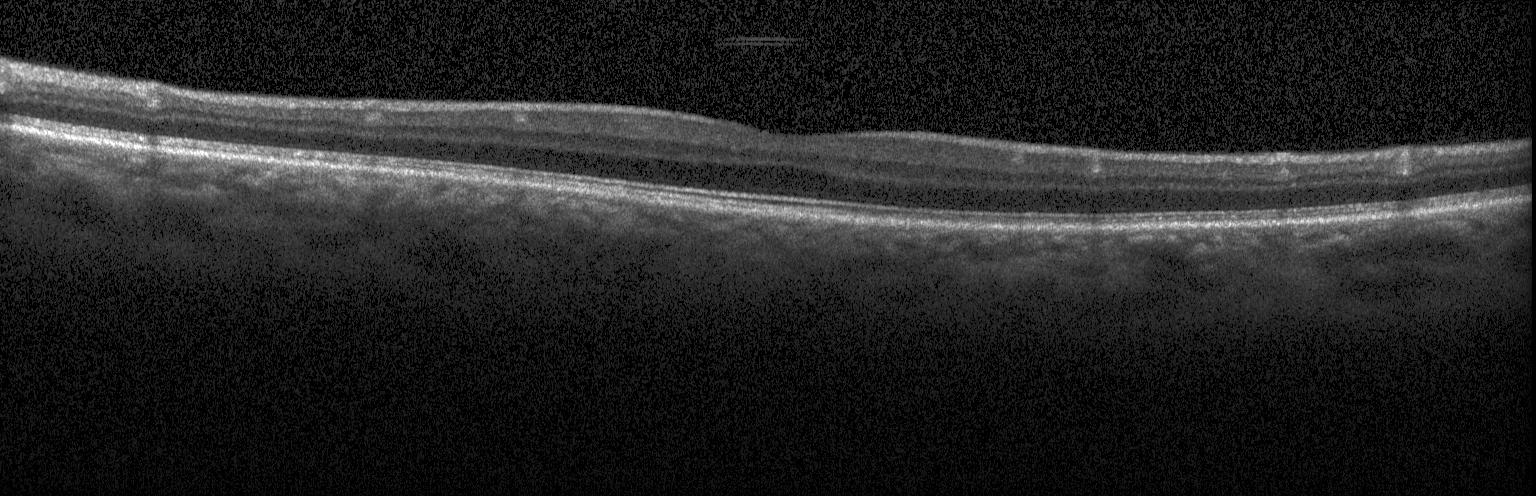

Centered on the fovea; retinal OCT cross-section; spectral-domain OCT — Diagnosis: no choroidal neovascularization, diabetic macular edema, or drusen.